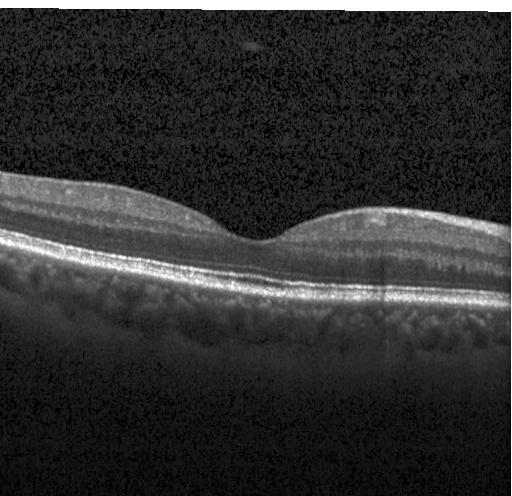

Optical coherence tomography B-scan; acquired on a Heidelberg Spectralis; macular scan
This B-scan demonstrates no evidence of choroidal neovascularization, diabetic macular edema, or drusen.